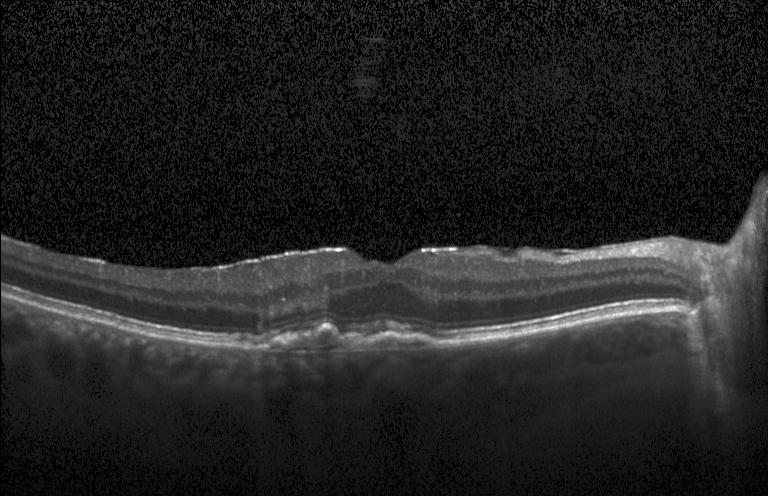
Centered on the fovea; instrument: Heidelberg Spectralis; optical coherence tomography scan; spectral-domain OCT. Finding: choroidal neovascularization.